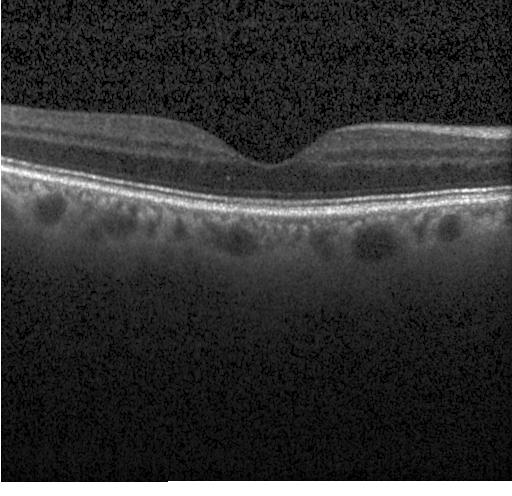

Impression: no evidence of choroidal neovascularization, diabetic macular edema, or drusen.